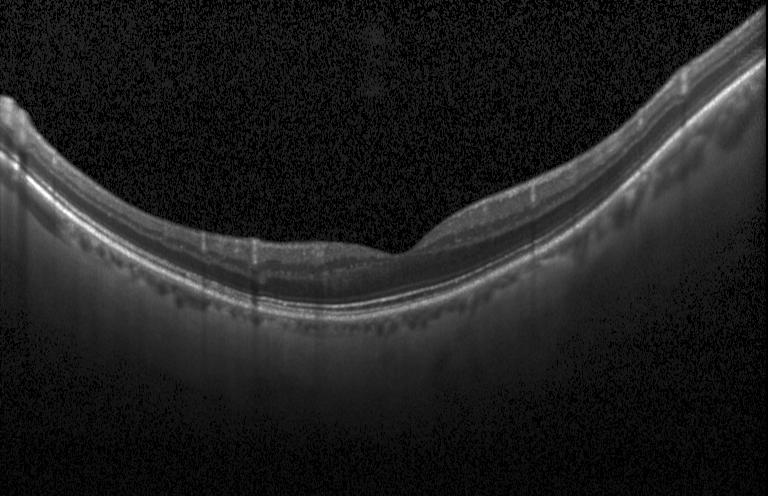 Assessment: no choroidal neovascularization, diabetic macular edema, or drusen.